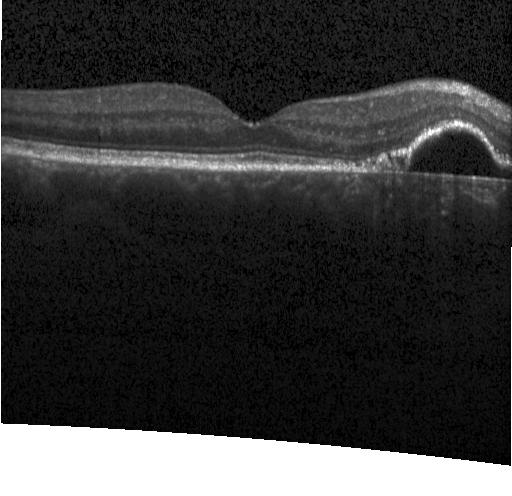
OCT B-scan showing choroidal neovascularization.